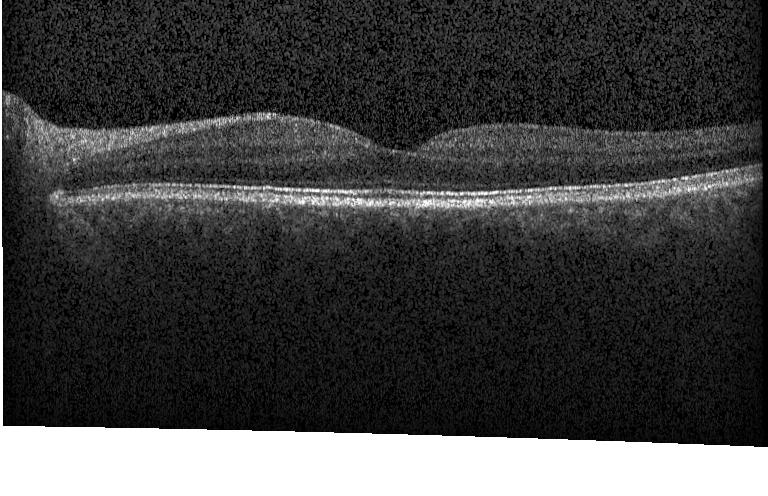
Spectral-domain OCT B-scan: no choroidal neovascularization, no diabetic macular edema, and no drusen.